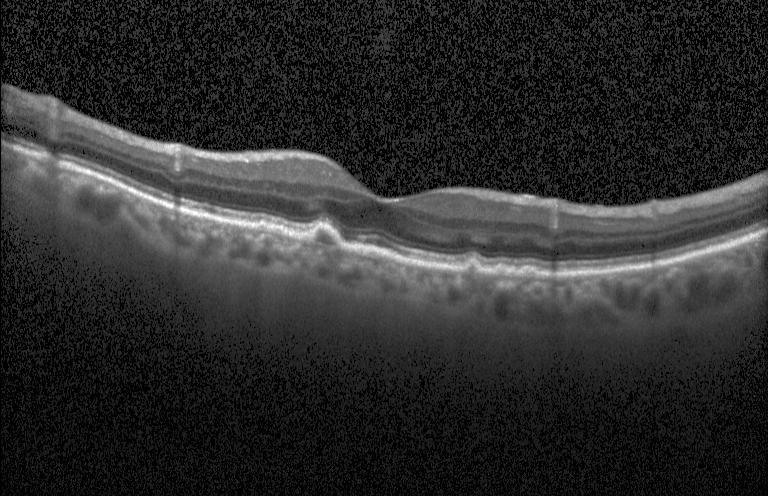

Diagnosis: sub-RPE drusenoid deposits.